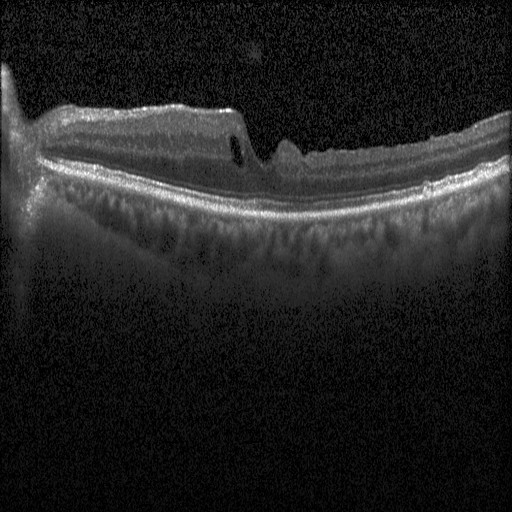

Dx: diabetic macular edema.